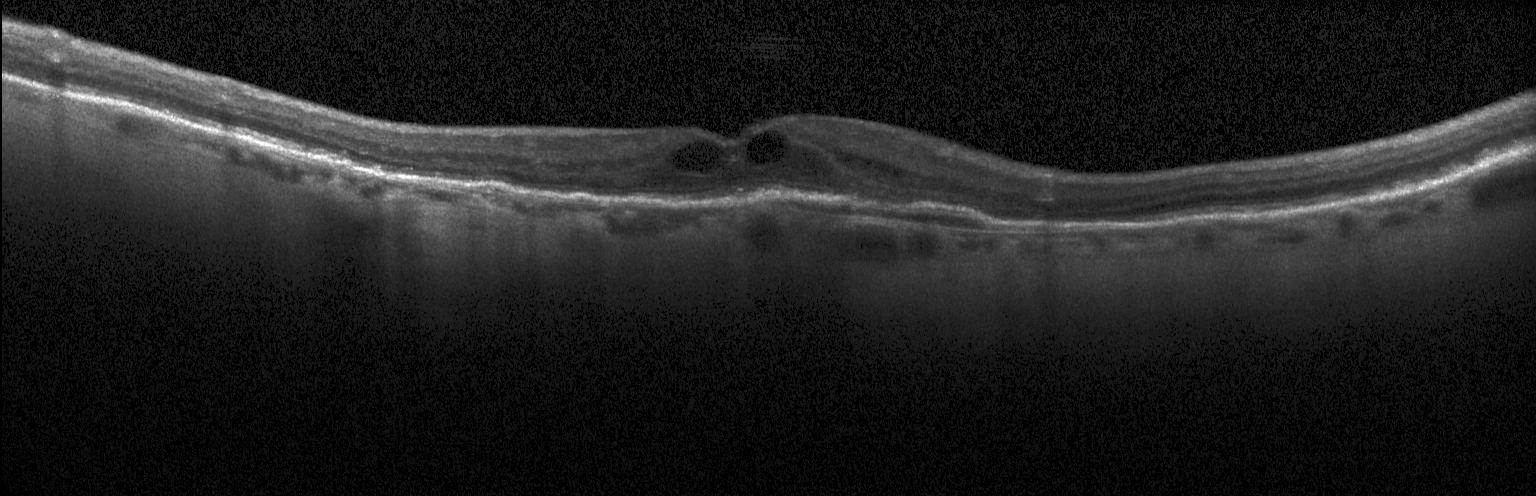
OCT B-scan showing choroidal neovascularization (CNV).